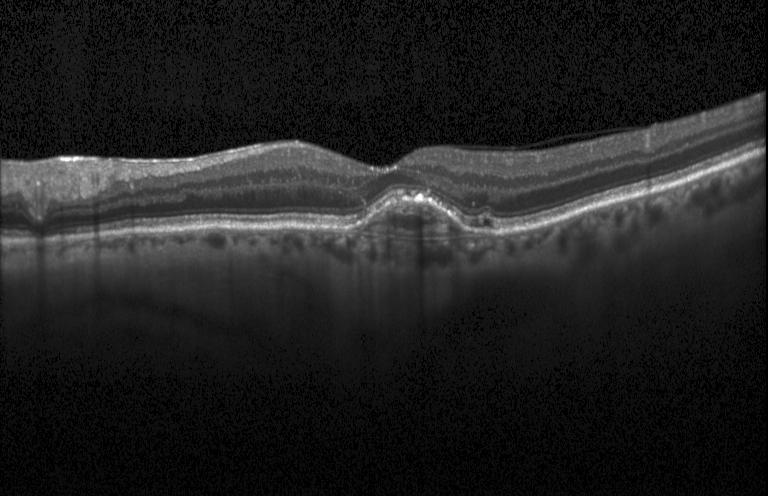 Retinal OCT B-scan.
Diagnosis: choroidal neovascularization.